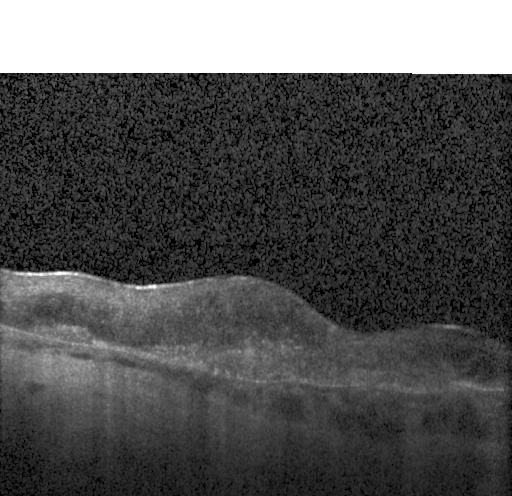
Optical coherence tomography scan, SD-OCT, Heidelberg Spectralis
This B-scan demonstrates a choroidal neovascular membrane.